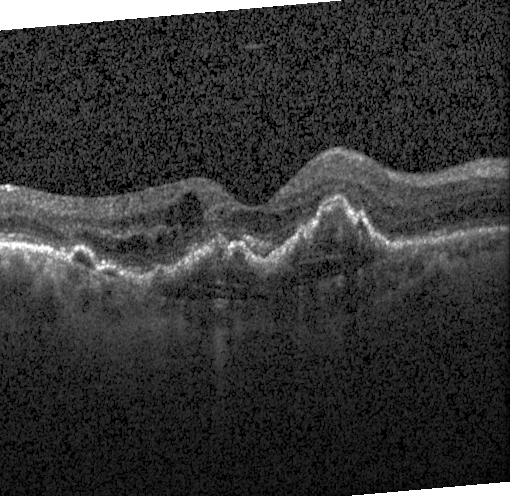
Centered on the fovea. Optical coherence tomography B-scan — Impression: choroidal neovascularization.